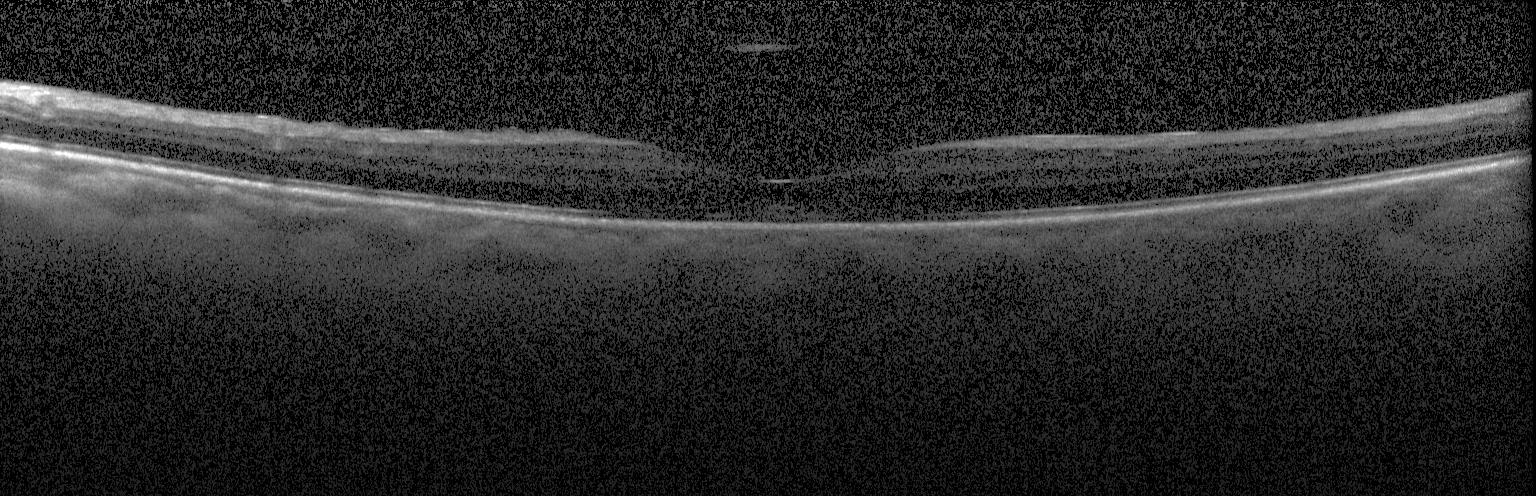

Optical coherence tomography B-scan — Diagnosis: no choroidal neovascularization, diabetic macular edema, or drusen.